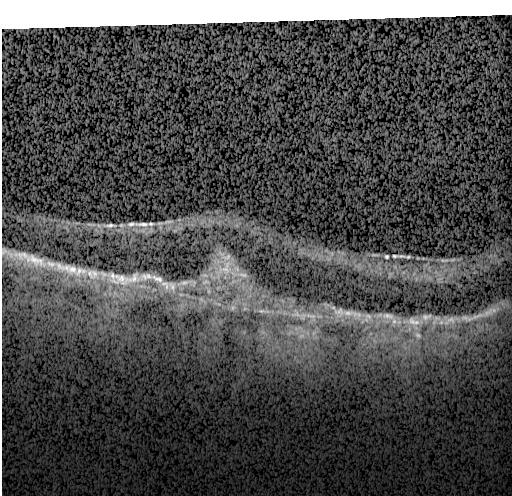
Heidelberg Spectralis; OCT B-scan; horizontal scan through the fovea.
A choroidal neovascular membrane.